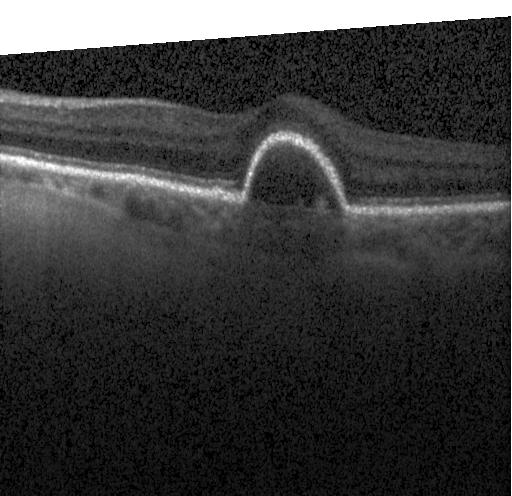

Impression: choroidal neovascularization.